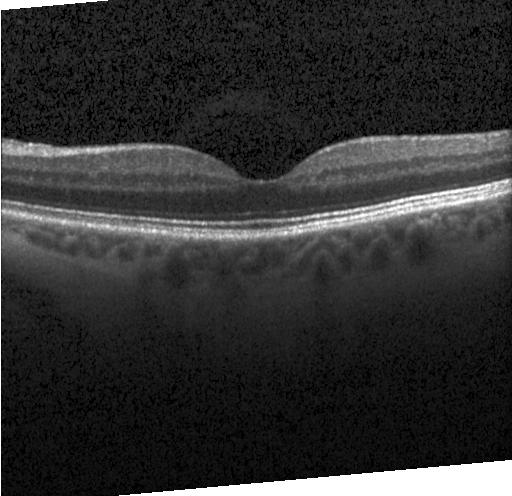

Assessment: no choroidal neovascularization, no diabetic macular edema, and no drusen.